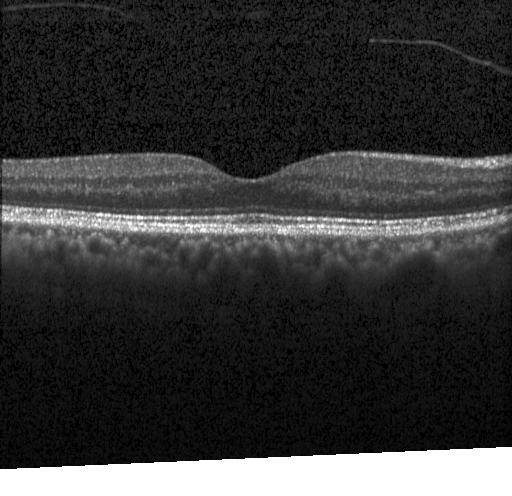 Optical coherence tomography scan — No choroidal neovascularization, diabetic macular edema, or drusen.